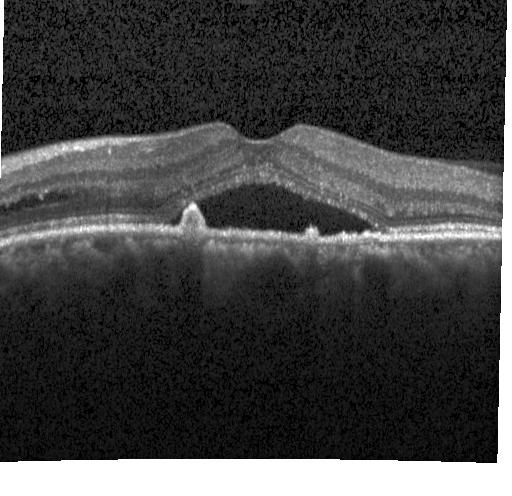 Acquired on a Heidelberg Spectralis; optical coherence tomography scan; spectral-domain optical coherence tomography; fovea-centered.
Dx: choroidal neovascularization.